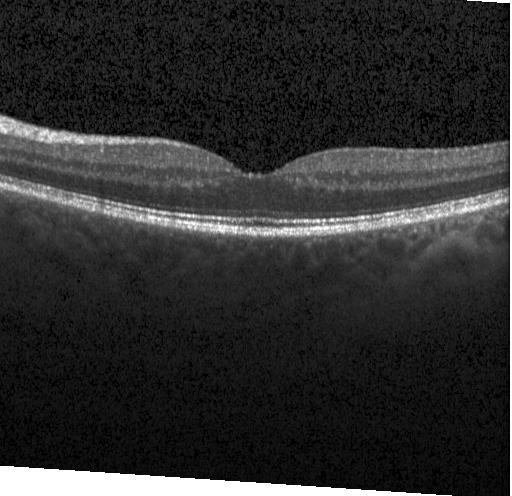 Optical coherence tomography scan.
Finding: no evidence of CNV, DME, or drusen.